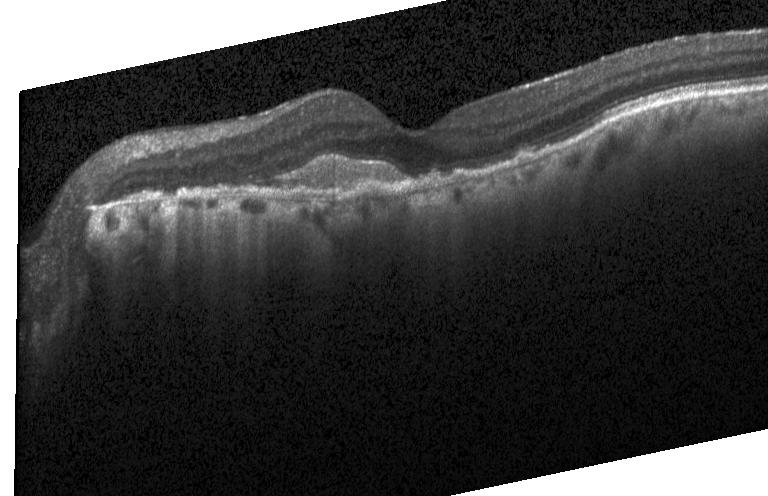 OCT B-scan showing a choroidal neovascular membrane.